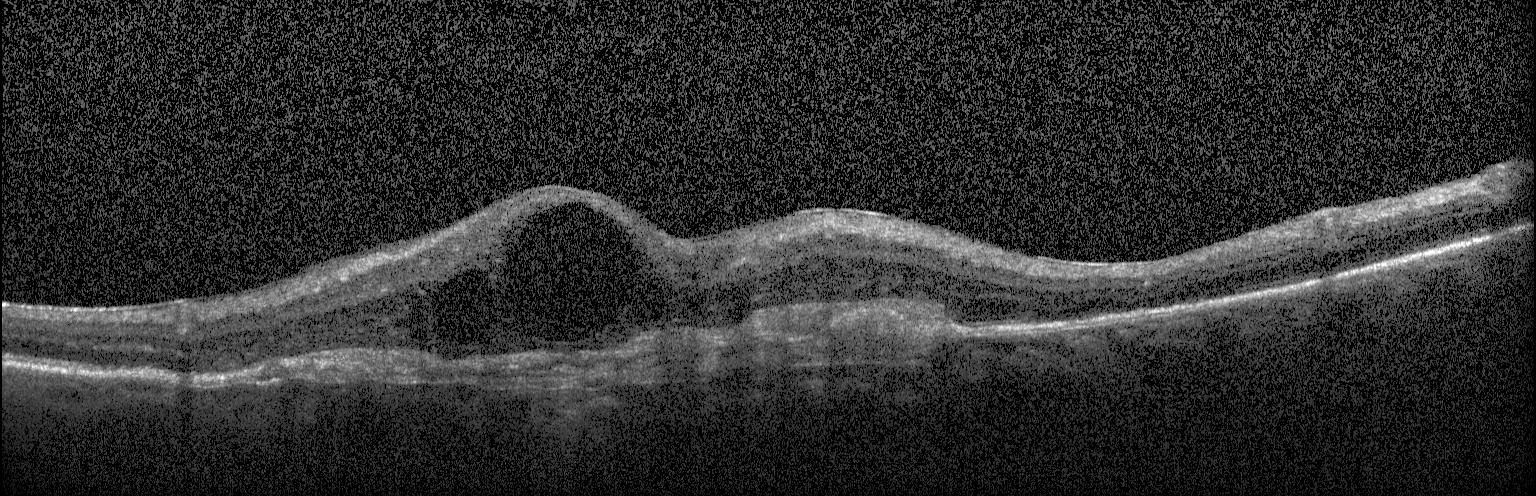 OCT finding: a choroidal neovascular membrane.